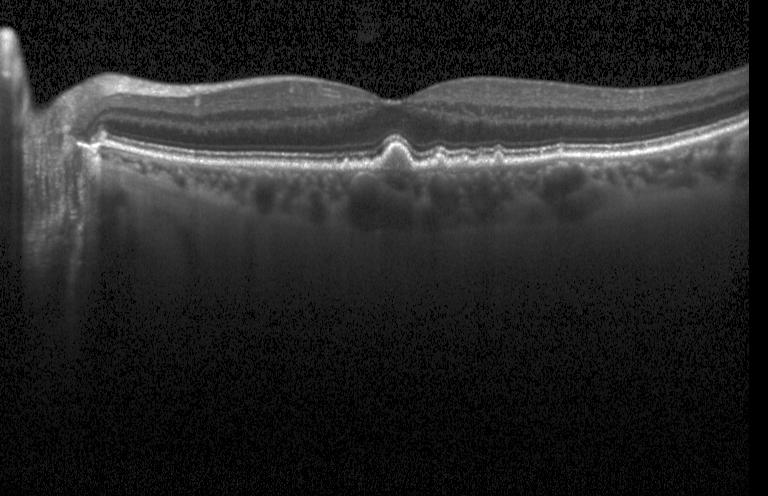
SD-OCT. Heidelberg Spectralis. Through the macula. Optical coherence tomography scan
Dx: drusen.